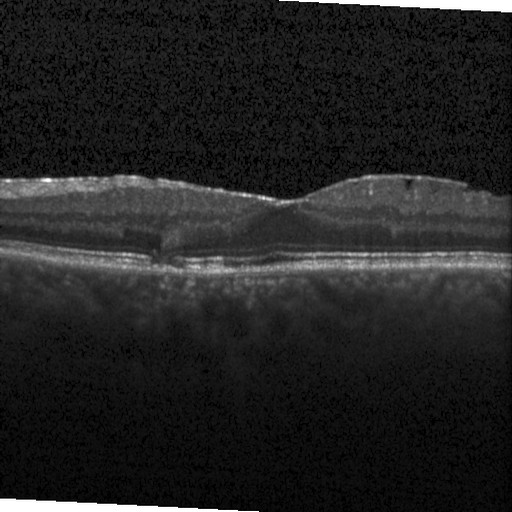 Heidelberg Spectralis OCT system; macular scan; spectral-domain OCT; optical coherence tomography B-scan
This B-scan demonstrates diabetic macular edema (DME).